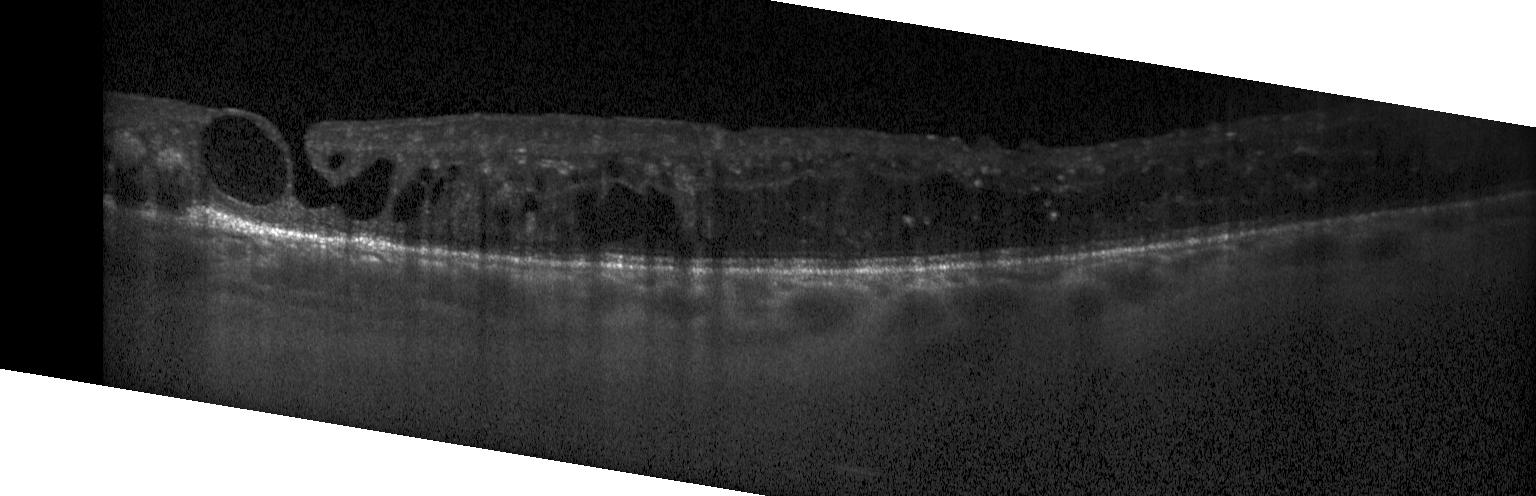 Spectral-domain OCT B-scan: diabetic macular edema (DME).